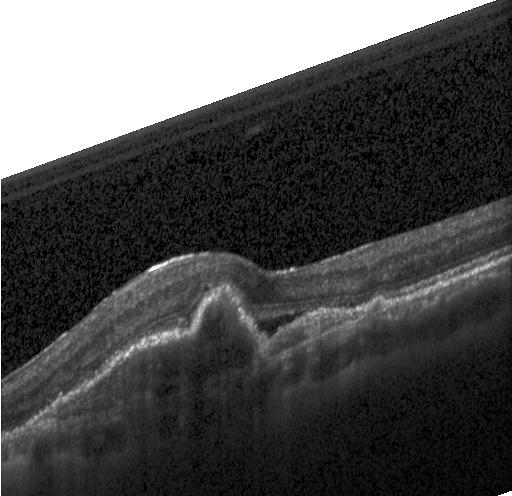

Retinal OCT B-scan — A choroidal neovascular membrane.